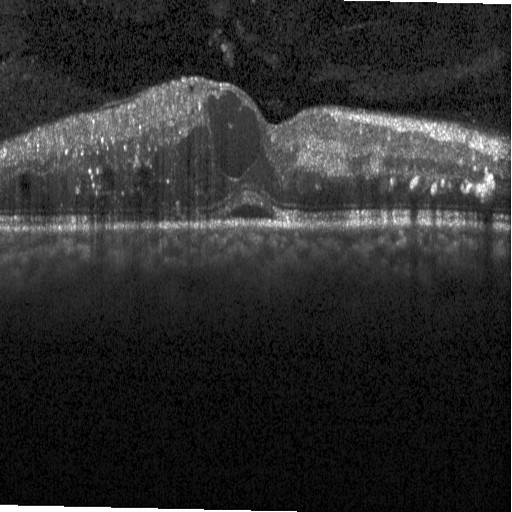

Retinal OCT cross-section showing diabetic macular edema.